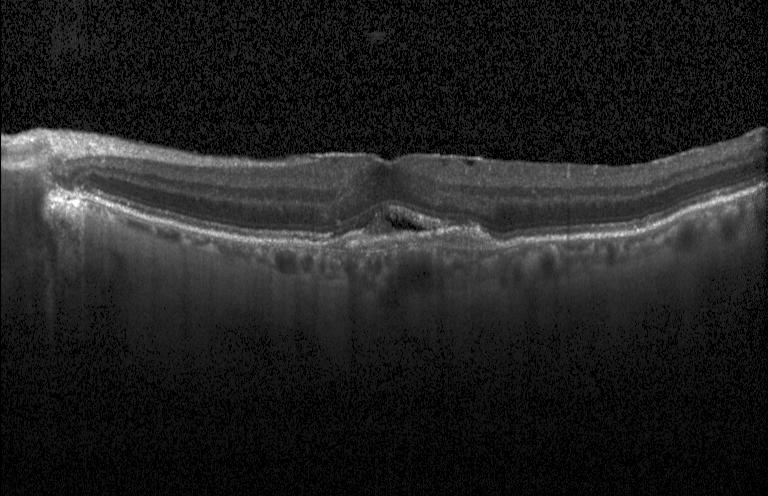
Heidelberg Spectralis, optical coherence tomography scan
Finding: a choroidal neovascular membrane.